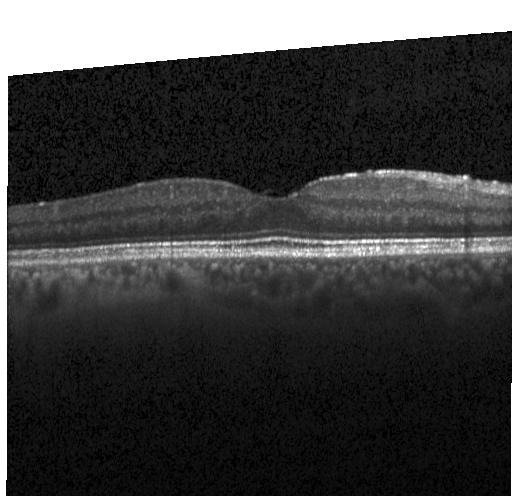

Instrument: Heidelberg Spectralis; spectral-domain OCT; macular scan; OCT line scan
Impression: no evidence of CNV, DME, or drusen.